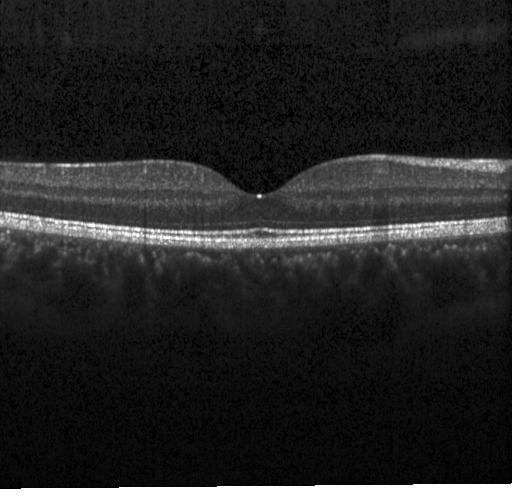 Spectral-domain OCT B-scan: neither CNV, DME, nor drusen.